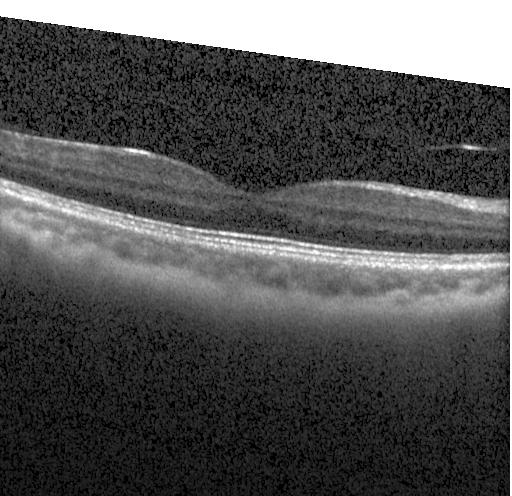

Instrument: Heidelberg Spectralis · optical coherence tomography scan · SD-OCT · macular scan. Finding: no choroidal neovascularization, no diabetic macular edema, and no drusen.